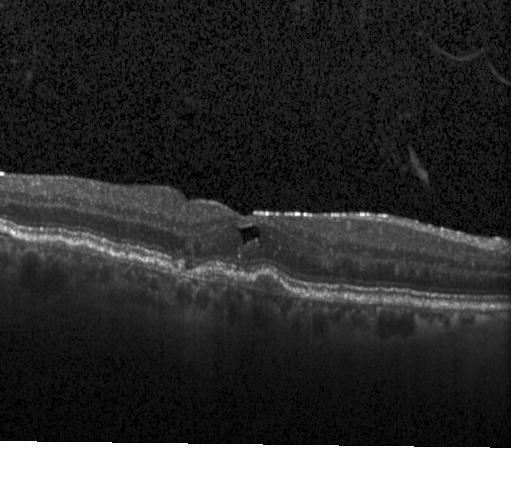

Retinal OCT B-scan; spectral-domain optical coherence tomography; fovea-centered. Finding: choroidal neovascularization (CNV).